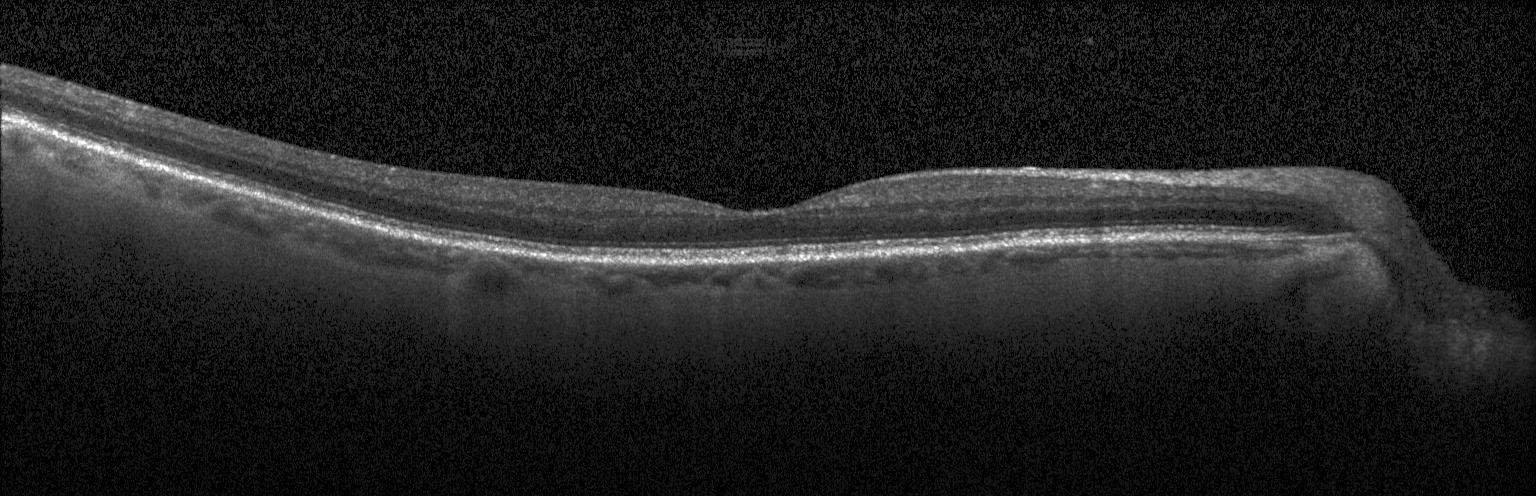

Optical coherence tomography B-scan. Diagnosis: no choroidal neovascularization, no diabetic macular edema, and no drusen.